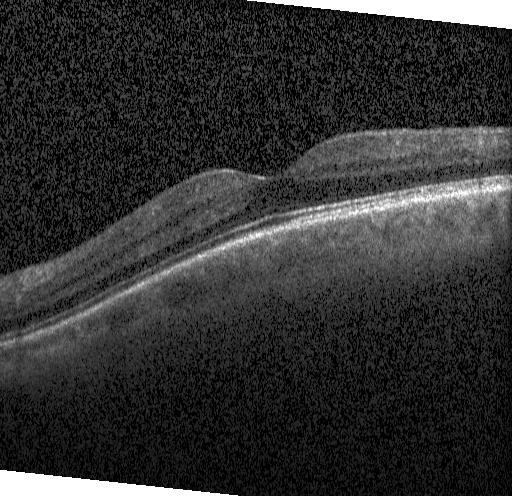
SD-OCT, OCT line scan
Finding: no choroidal neovascularization, diabetic macular edema, or drusen.